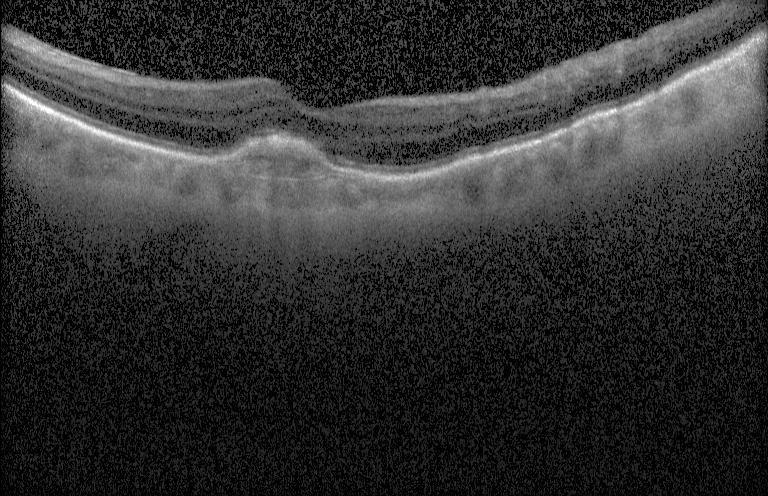 OCT finding: CNV.